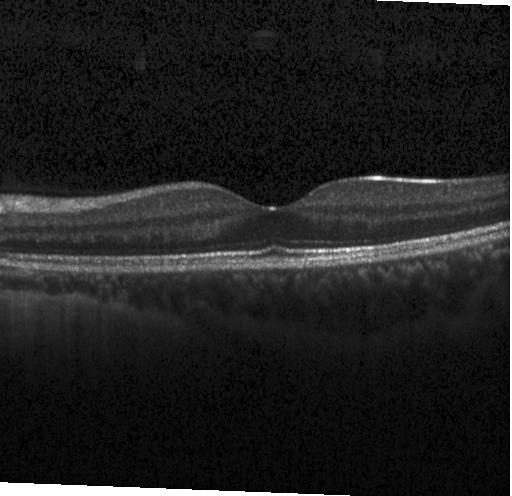

Heidelberg Spectralis; optical coherence tomography B-scan; spectral-domain OCT — No choroidal neovascularization, no diabetic macular edema, and no drusen.